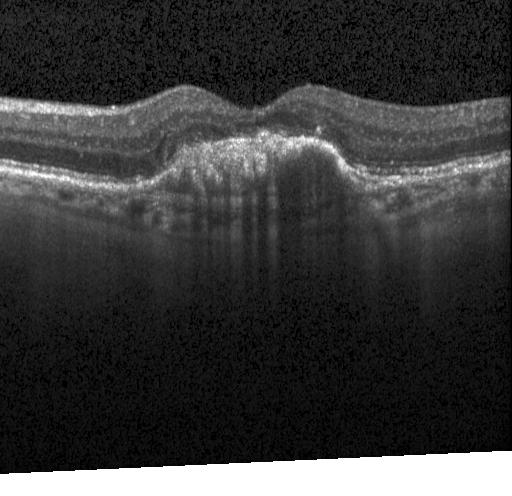 Finding: choroidal neovascularization (CNV).